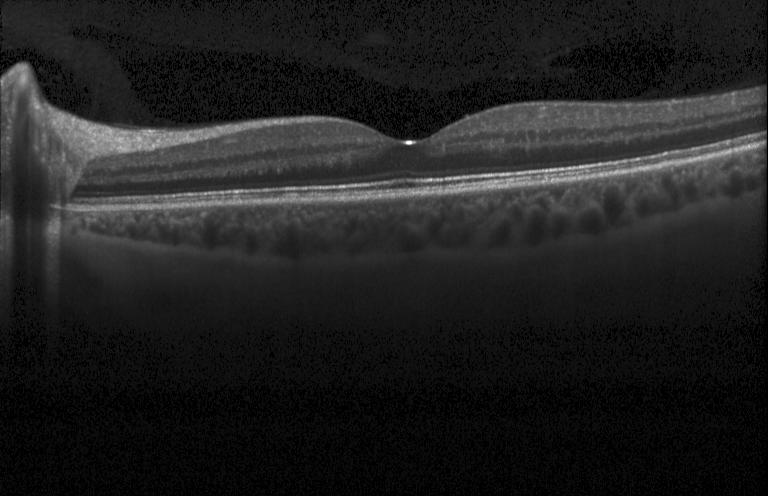

Macular OCT: neither CNV, DME, nor drusen.